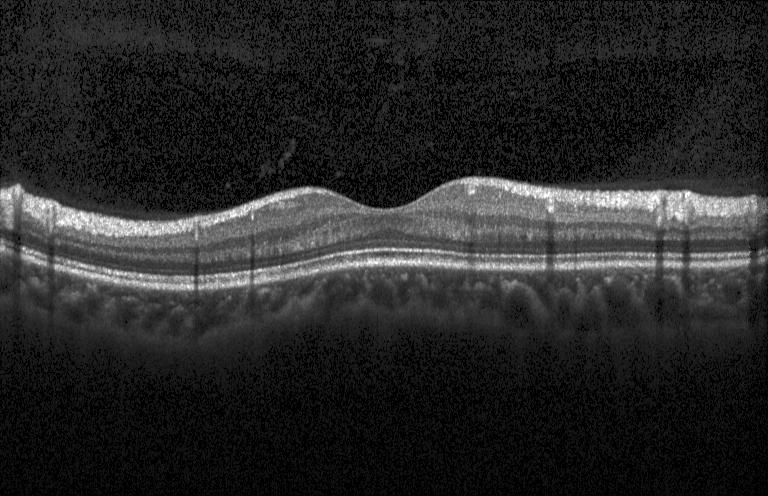 Retinal OCT B-scan. Impression: no choroidal neovascularization, no diabetic macular edema, and no drusen.